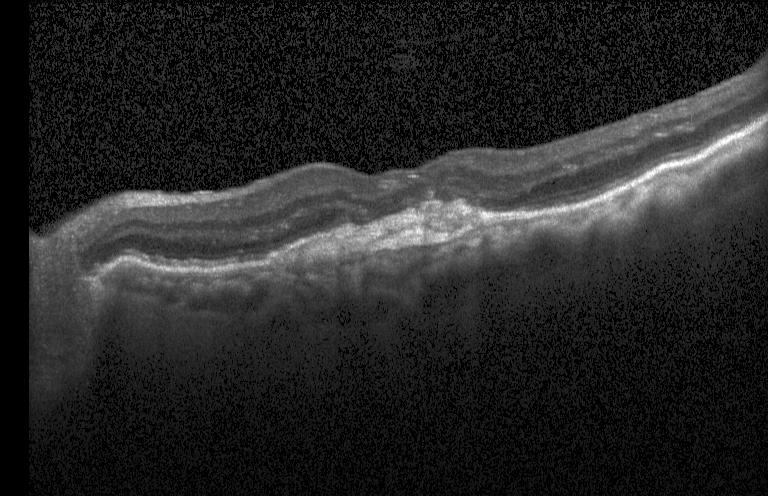 OCT B-scan, instrument: Heidelberg Spectralis, horizontal scan through the fovea, spectral-domain OCT.
This B-scan demonstrates a choroidal neovascular membrane.